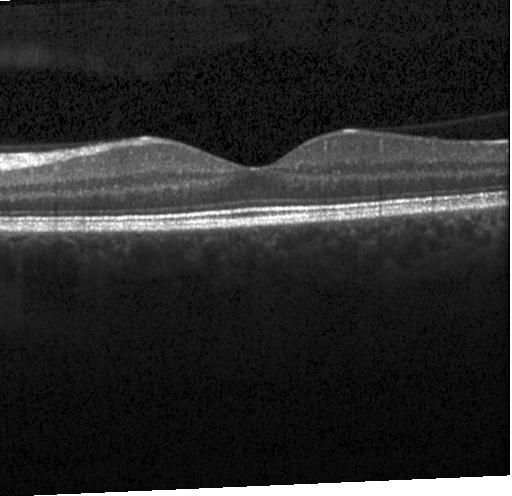

Spectral-domain OCT, macular scan, retinal OCT cross-section.
Finding: no evidence of CNV, DME, or drusen.